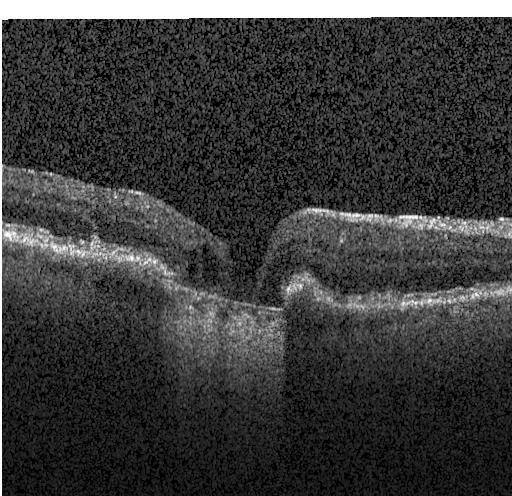 OCT B-scan; SD-OCT; instrument: Heidelberg Spectralis; centered on the fovea
Dx: a choroidal neovascular membrane.